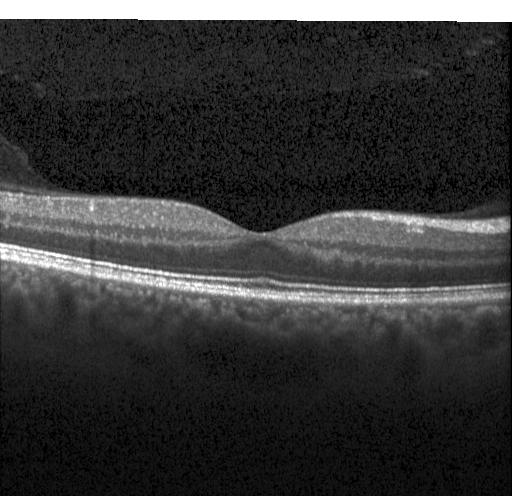
Retinal OCT cross-section showing no CNV, no DME, and no drusen.